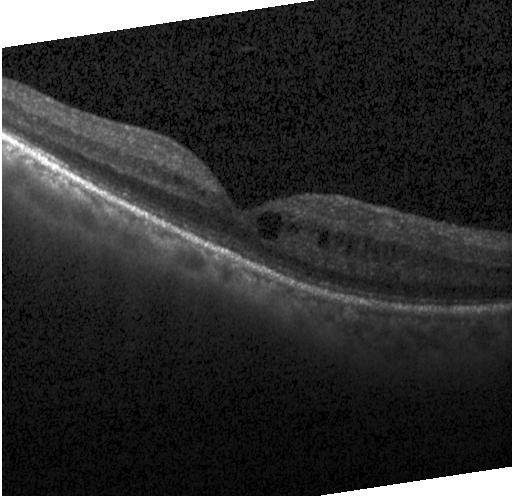 Spectral-domain OCT · OCT line scan · horizontal scan through the fovea.
The scan shows diabetic macular edema (DME).